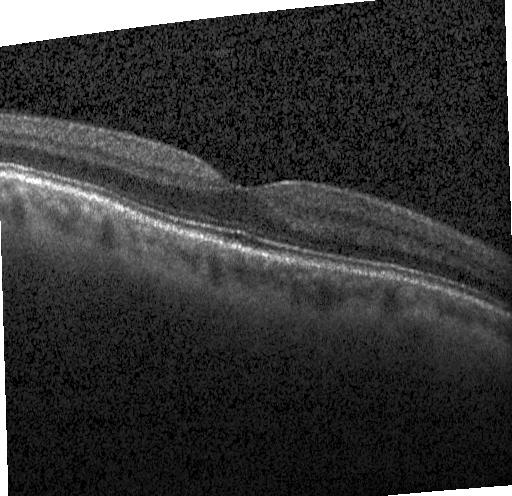
Dx: no choroidal neovascularization, no diabetic macular edema, and no drusen.